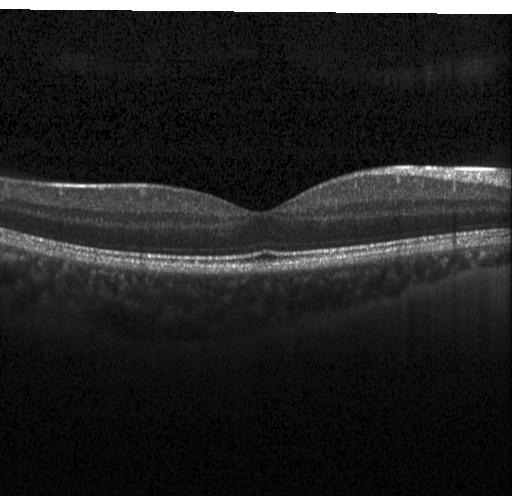

Optical coherence tomography scan — Neither CNV, DME, nor drusen.